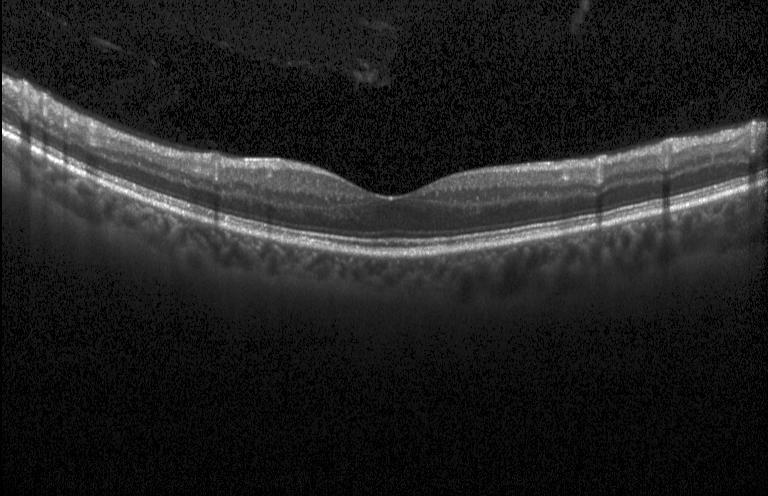 Optical coherence tomography scan · SD-OCT.
Dx: neither choroidal neovascularization, diabetic macular edema, nor drusen.